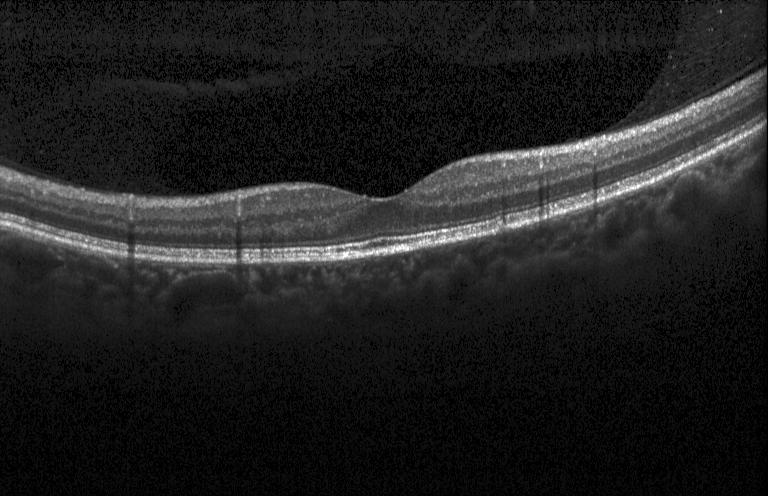

OCT finding: no choroidal neovascularization, diabetic macular edema, or drusen.